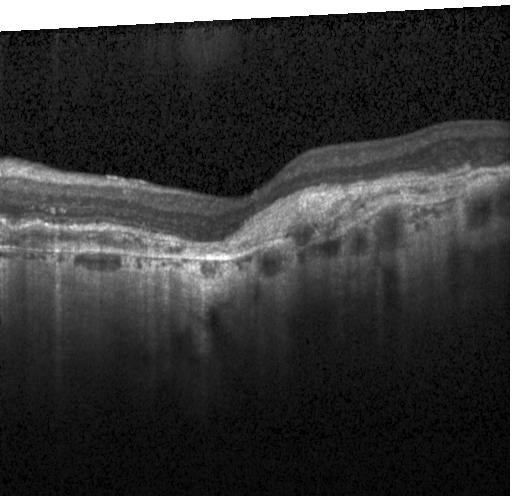

Dx: a choroidal neovascular membrane.